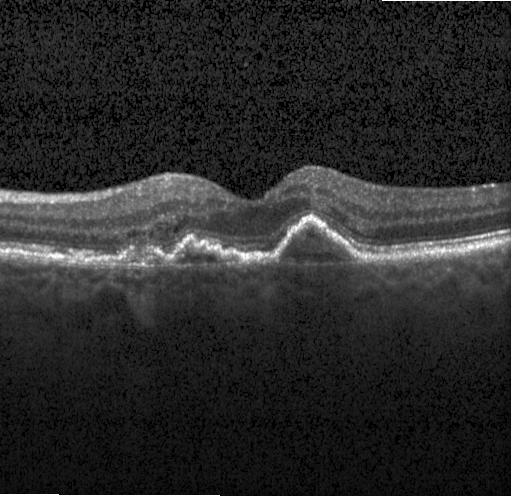 Optical coherence tomography B-scan
The scan shows choroidal neovascularization.